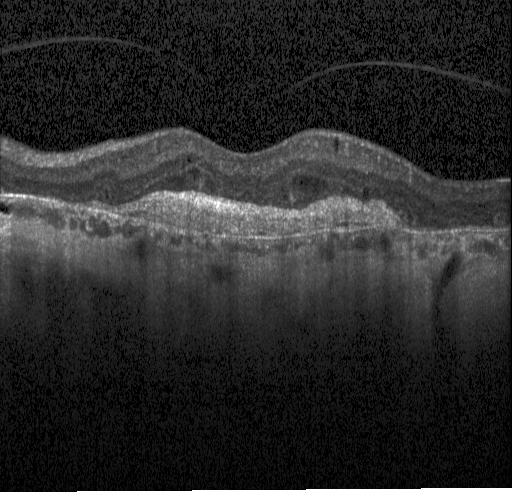
Retinal OCT B-scan — Impression: a choroidal neovascular membrane.